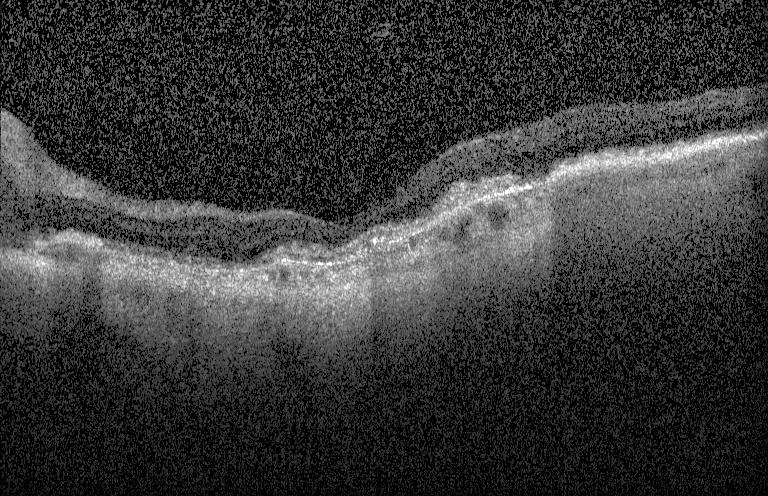

Optical coherence tomography scan; SD-OCT; Heidelberg Spectralis.
The scan shows a choroidal neovascular membrane.